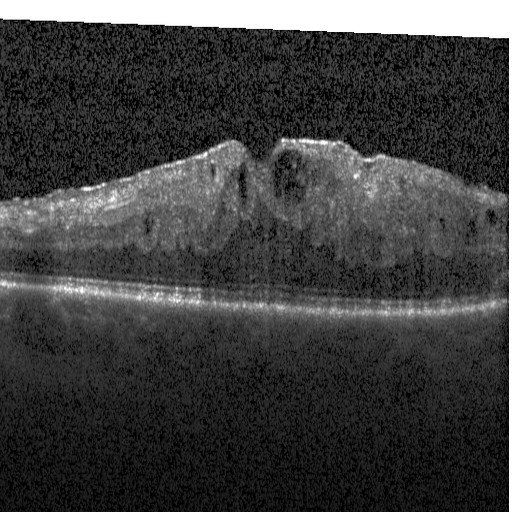
This B-scan demonstrates diabetic macular edema (DME).